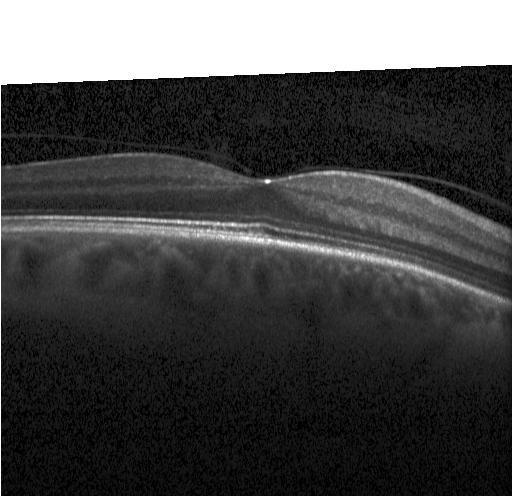

Spectral-domain optical coherence tomography, OCT B-scan
No CNV, DME, or drusen.